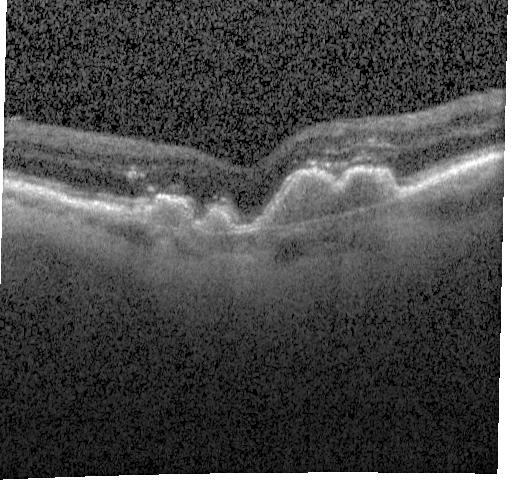
Assessment: choroidal neovascularization.